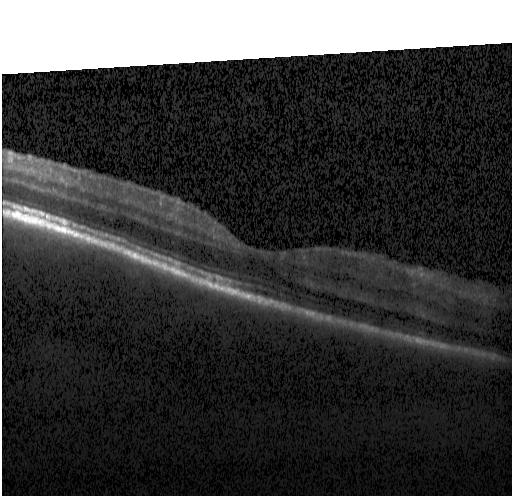
Spectral-domain optical coherence tomography. OCT B-scan. No evidence of choroidal neovascularization, diabetic macular edema, or drusen.